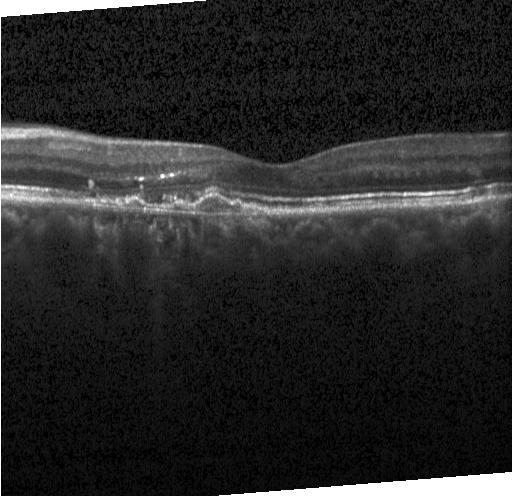 Optical coherence tomography scan — A choroidal neovascular membrane.